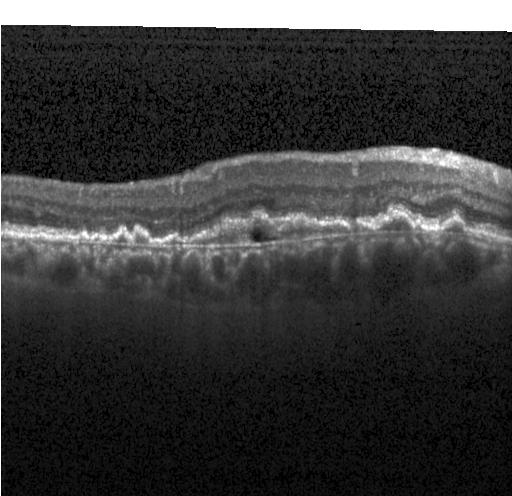 OCT B-scan. Spectral-domain optical coherence tomography. Through the macula — Impression: choroidal neovascularization.